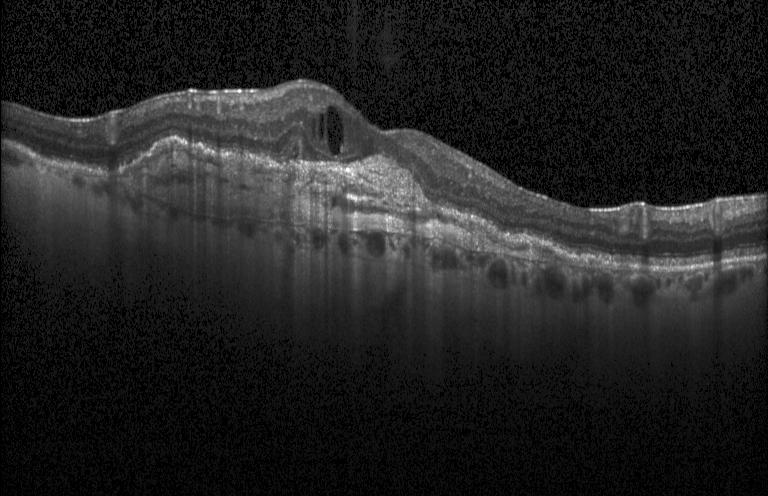

Retinal OCT cross-section
Diagnosis: CNV.